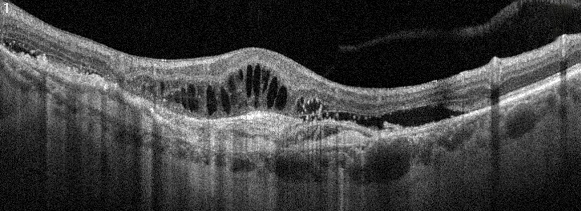

Optical coherence tomography scan; right eye; fovea-centered; Optovue Avanti RTVue XR.
Age-related macular degeneration (AMD).